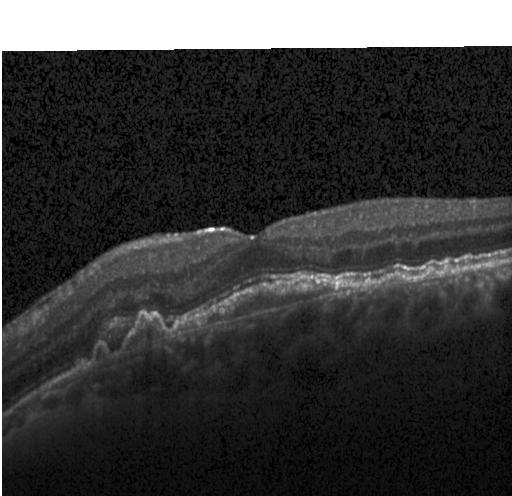
OCT B-scan. Diagnosis: a choroidal neovascular membrane.